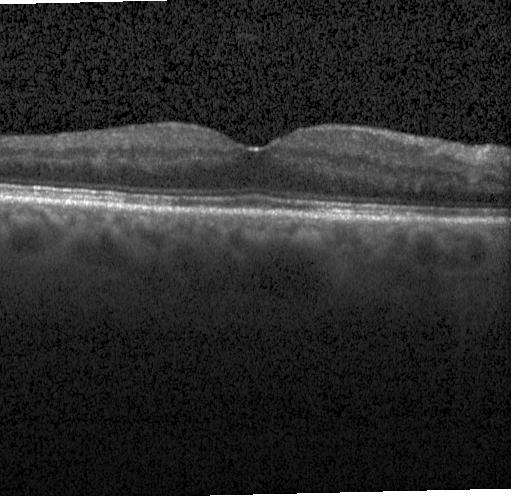
OCT B-scan, spectral-domain OCT, Heidelberg Spectralis. Dx: neither choroidal neovascularization, diabetic macular edema, nor drusen.